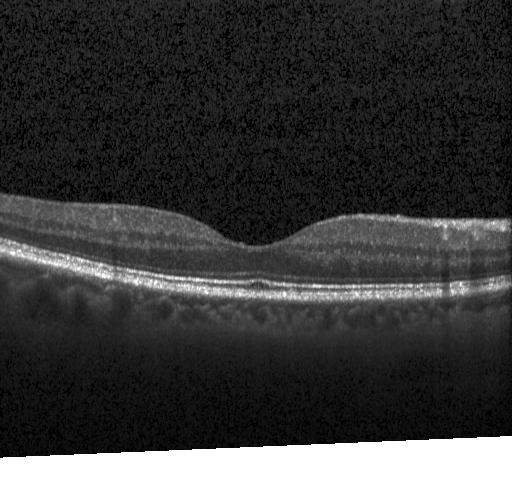
Dx: no evidence of choroidal neovascularization, diabetic macular edema, or drusen.